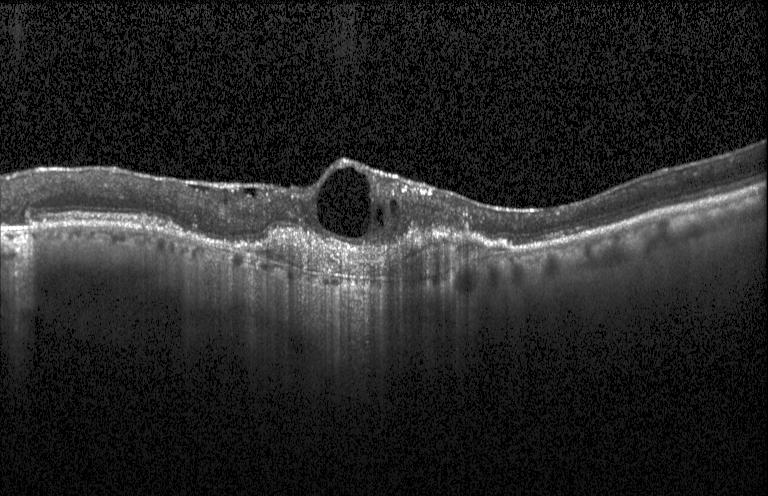

Impression: CNV.